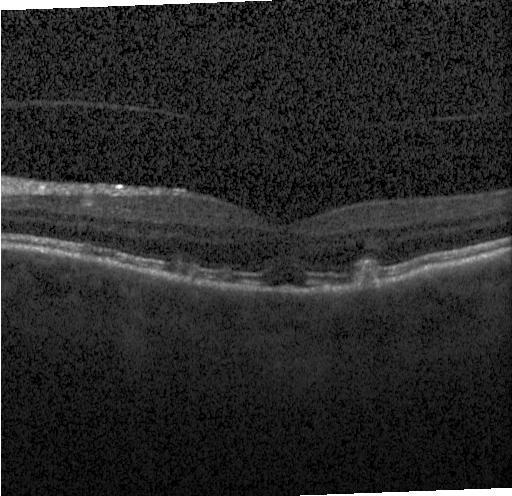

OCT finding: drusen.